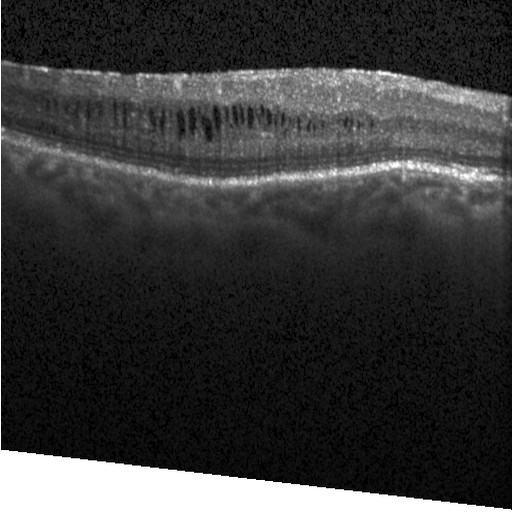 OCT finding: DME.